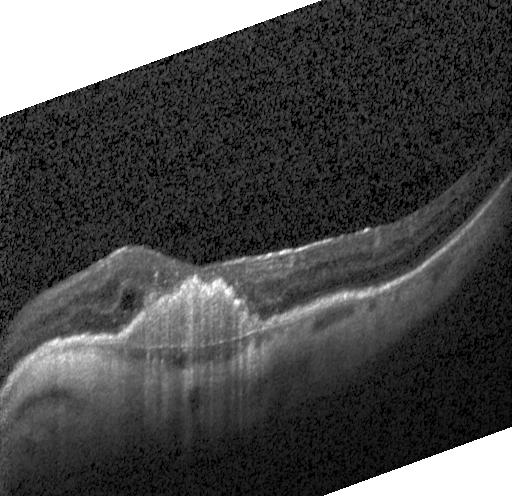

Retinal OCT cross-section showing a choroidal neovascular membrane.